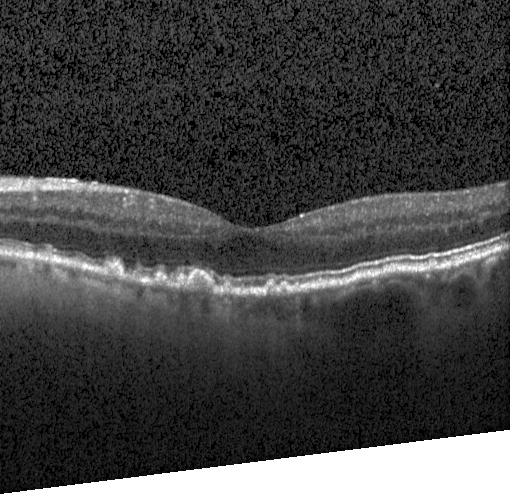

Finding: multiple drusen.